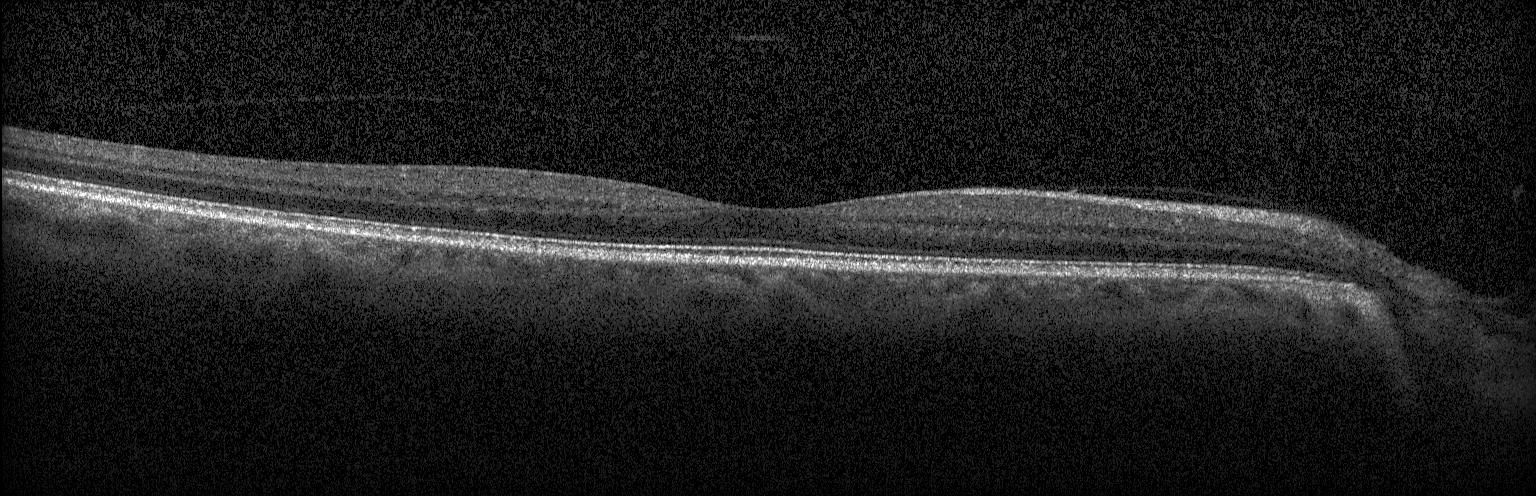

OCT line scan · centered on the fovea. This B-scan demonstrates no choroidal neovascularization, diabetic macular edema, or drusen.